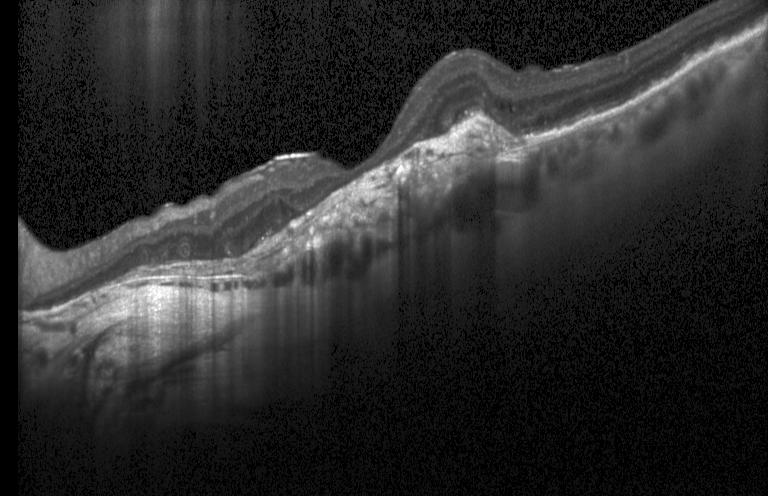

Macular OCT: a choroidal neovascular membrane.